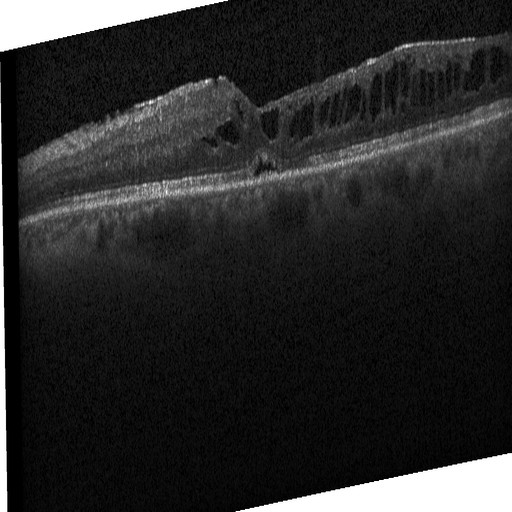 Acquired on a Heidelberg Spectralis; through the macula; optical coherence tomography B-scan — OCT finding: DME.